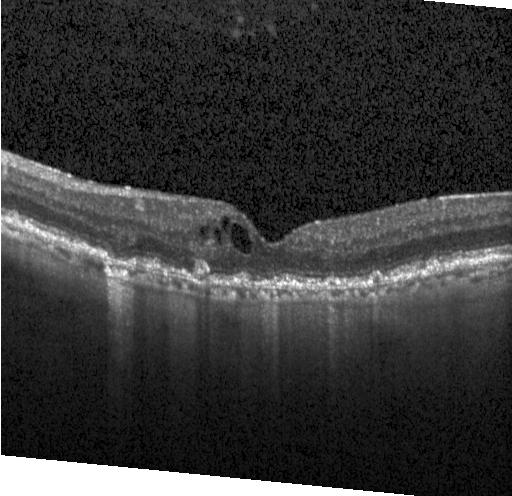

Optical coherence tomography scan, Heidelberg Spectralis. The scan shows CNV.